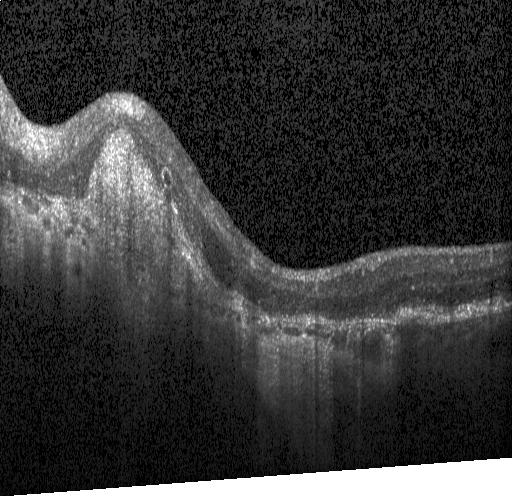
Spectral-domain OCT · OCT B-scan · horizontal scan through the fovea · Heidelberg Spectralis. A choroidal neovascular membrane.